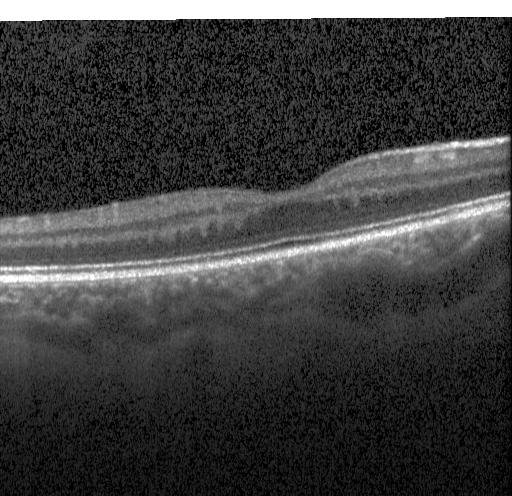

Assessment: neither CNV, DME, nor drusen.